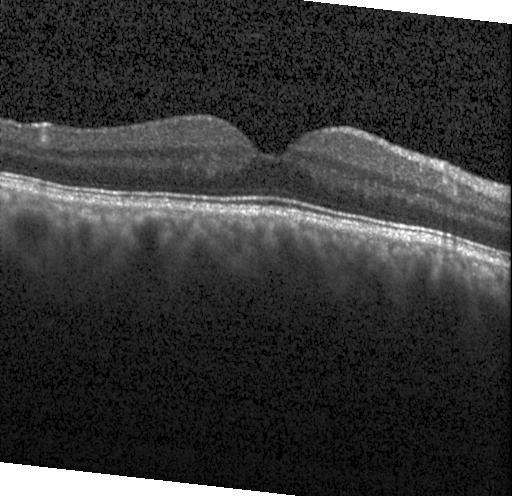
Fovea-centered, spectral-domain OCT, OCT line scan
The scan shows no evidence of CNV, DME, or drusen.